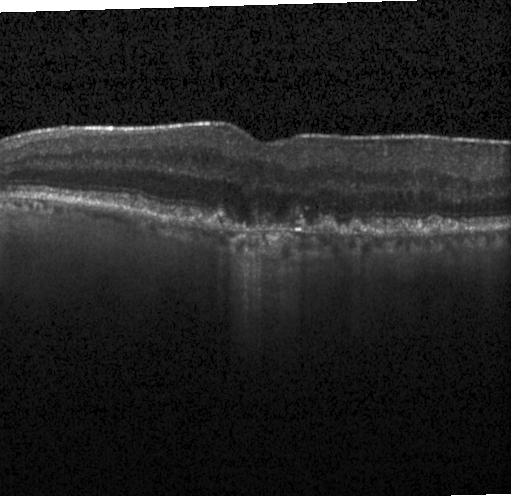
Finding: choroidal neovascularization (CNV).